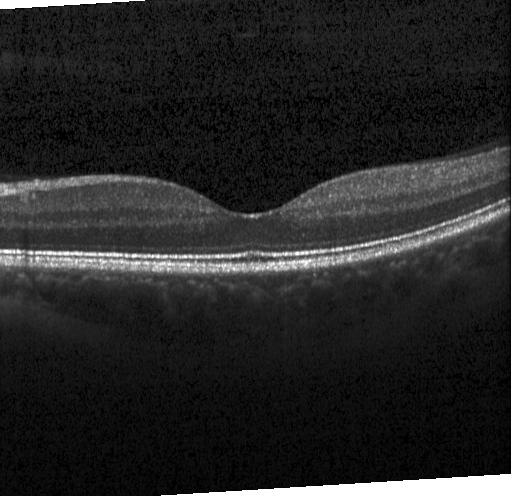
Retinal OCT B-scan — No evidence of choroidal neovascularization, diabetic macular edema, or drusen.